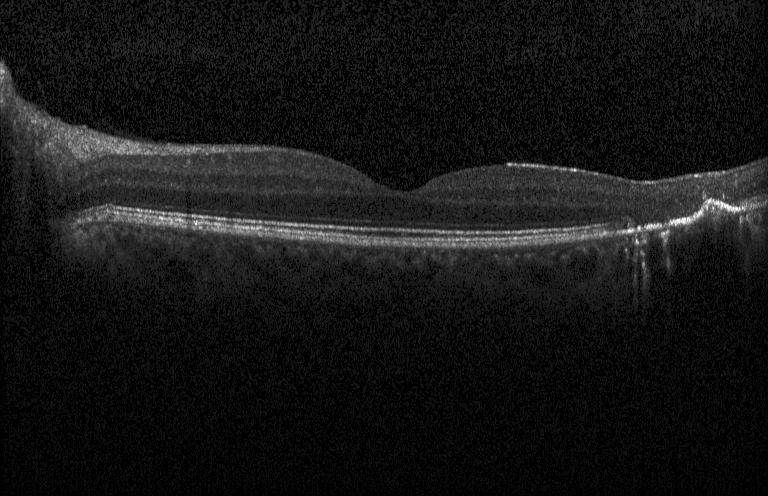
Diagnosis: a choroidal neovascular membrane.